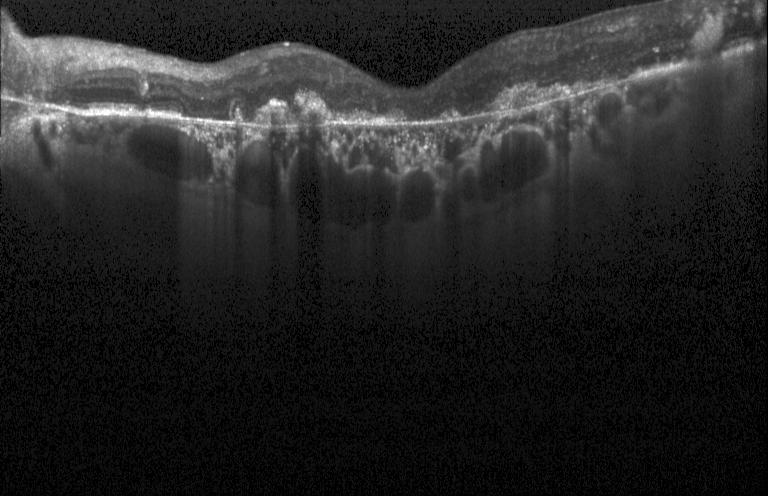

Optical coherence tomography scan.
Diagnosis: a choroidal neovascular membrane.